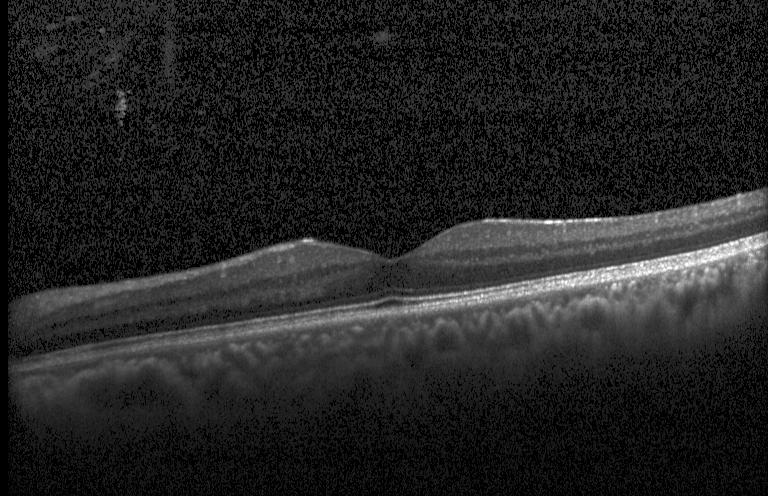

Finding: no choroidal neovascularization, no diabetic macular edema, and no drusen.